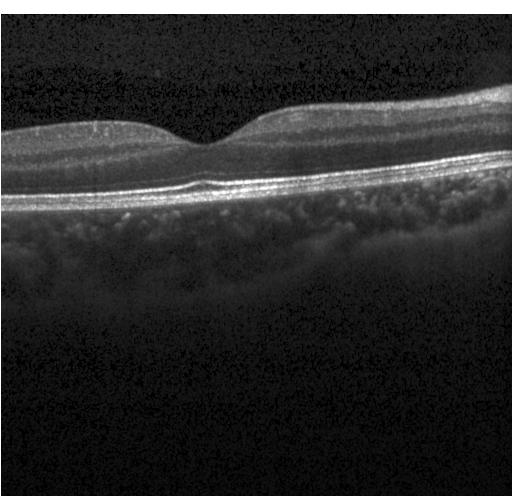
Neither choroidal neovascularization, diabetic macular edema, nor drusen.